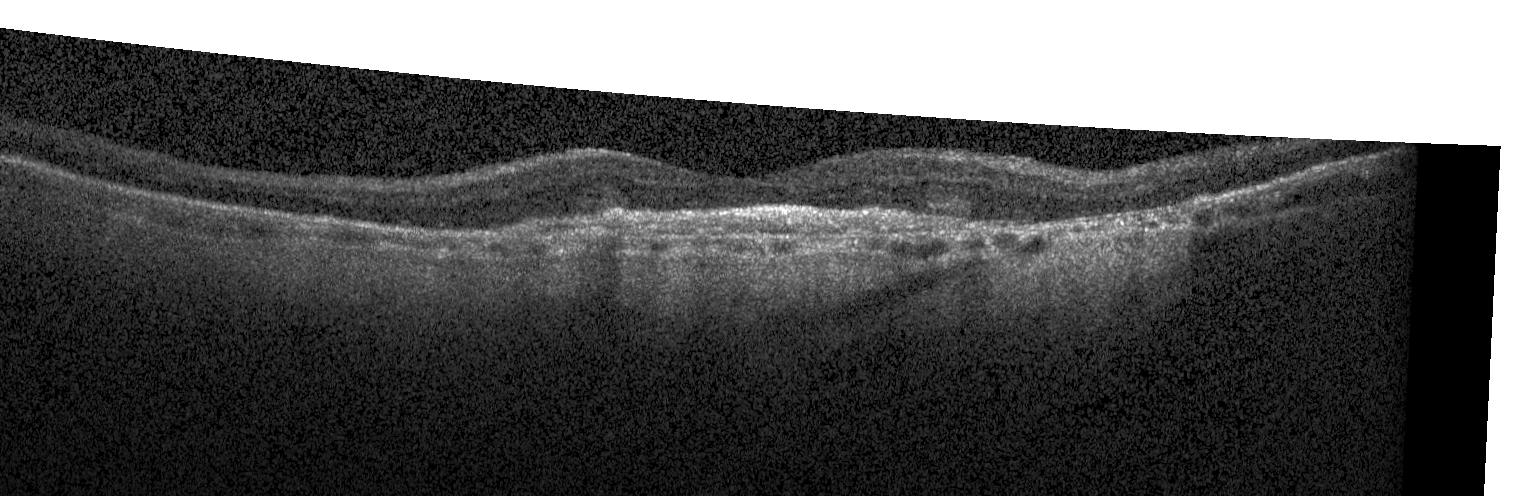
Macular OCT: choroidal neovascularization (CNV).